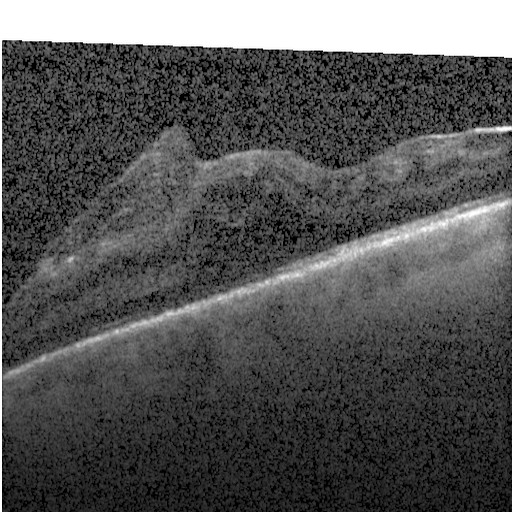

This B-scan demonstrates DME.